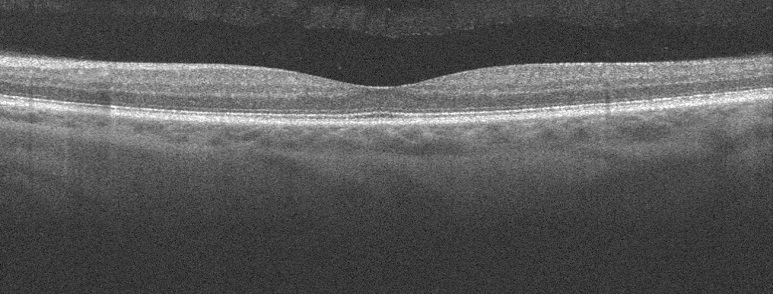
Optovue Avanti RTVue XR, fovea-centered, retinal OCT cross-section.
Diagnosis: no AMD, DME, ERM, RAO, RVO, or VID.